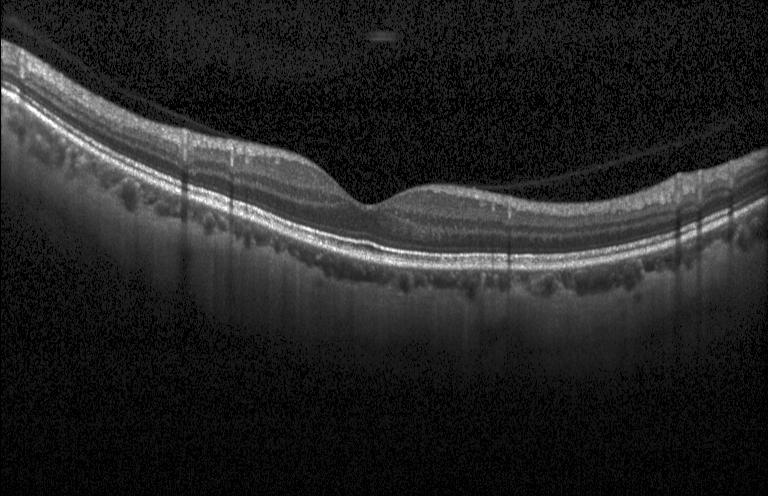

Optical coherence tomography B-scan · spectral-domain optical coherence tomography. OCT finding: no CNV, no DME, and no drusen.